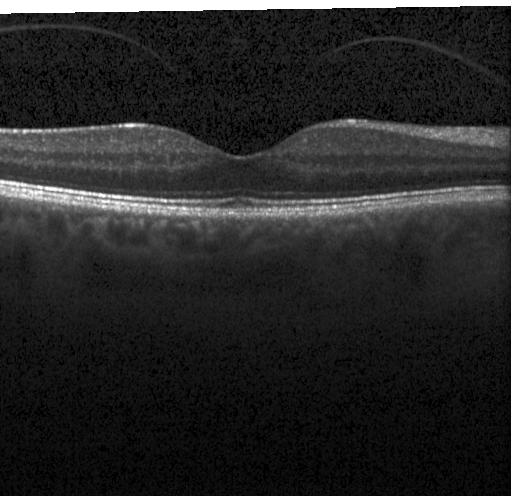
Retinal OCT cross-section showing no CNV, DME, or drusen.